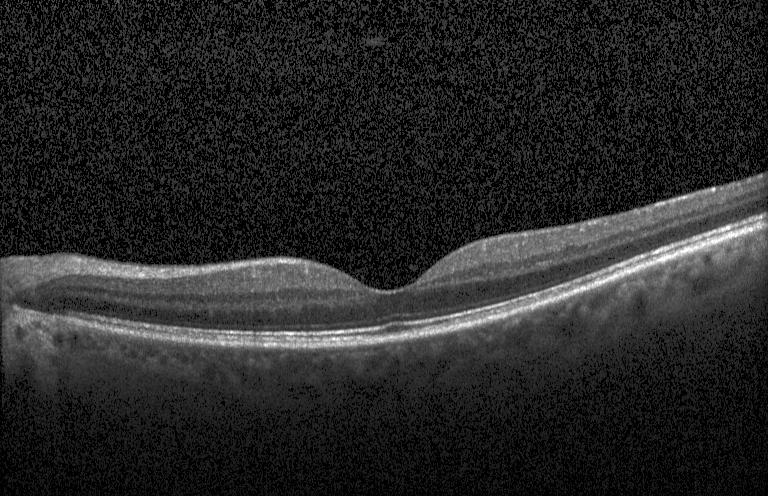
SD-OCT · Heidelberg Spectralis OCT system · OCT B-scan · fovea-centered.
Impression: no choroidal neovascularization, no diabetic macular edema, and no drusen.